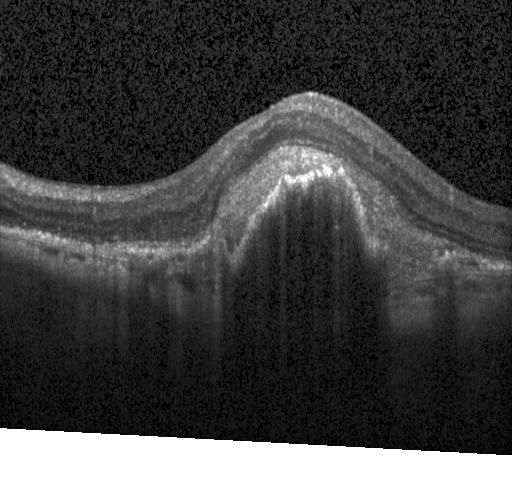

Spectral-domain OCT B-scan: a choroidal neovascular membrane.